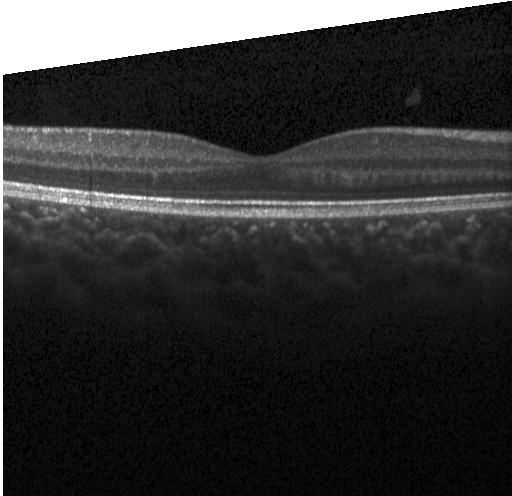 OCT B-scan. Acquired on a Heidelberg Spectralis. Spectral-domain optical coherence tomography — Finding: no CNV, DME, or drusen.